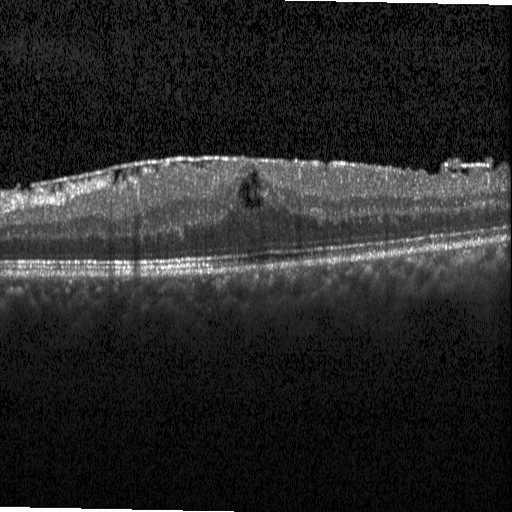

Macular OCT demonstrating DME.